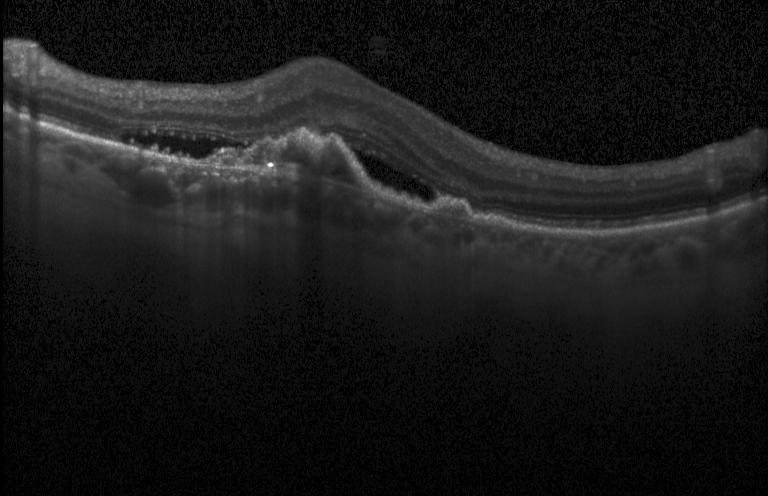
OCT scan showing a choroidal neovascular membrane.